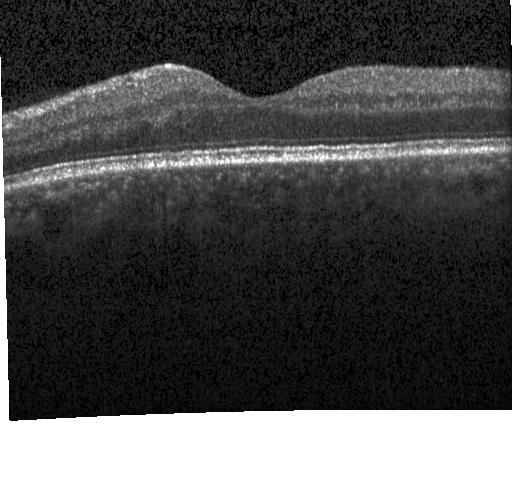 The scan shows no evidence of choroidal neovascularization, diabetic macular edema, or drusen.